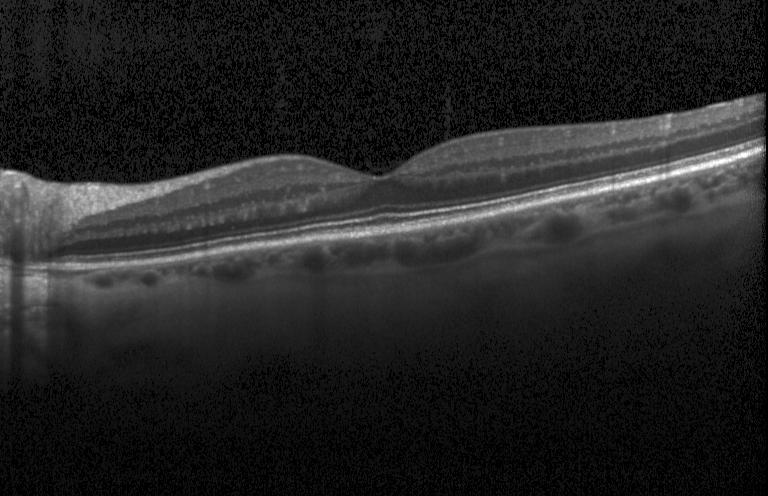

SD-OCT; retinal OCT cross-section.
Diagnosis: no evidence of CNV, DME, or drusen.